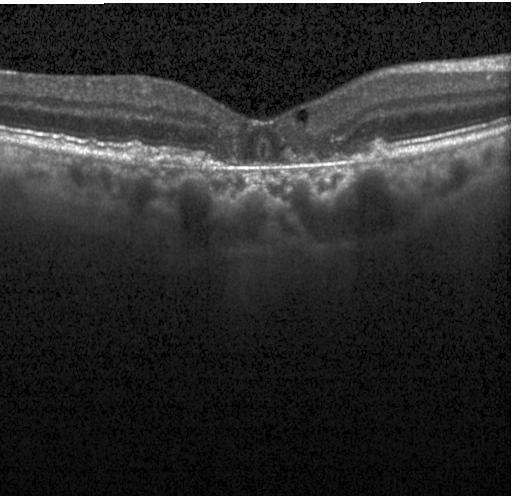
Diagnosis: choroidal neovascularization (CNV).